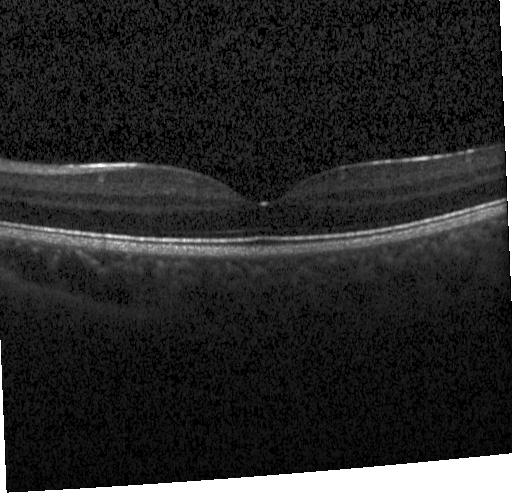 OCT finding: no choroidal neovascularization, no diabetic macular edema, and no drusen.